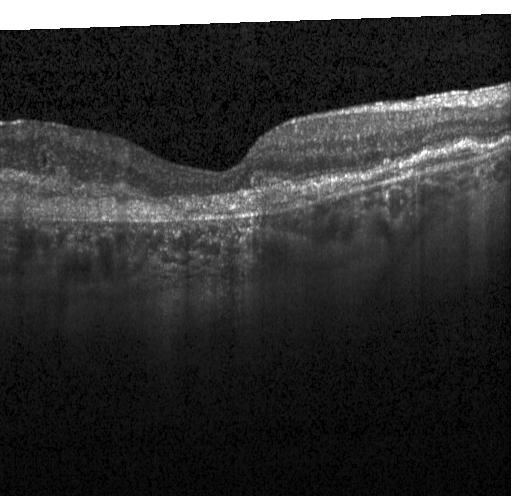

OCT B-scan; macular scan; Heidelberg Spectralis OCT system; spectral-domain optical coherence tomography.
Macular OCT: CNV.